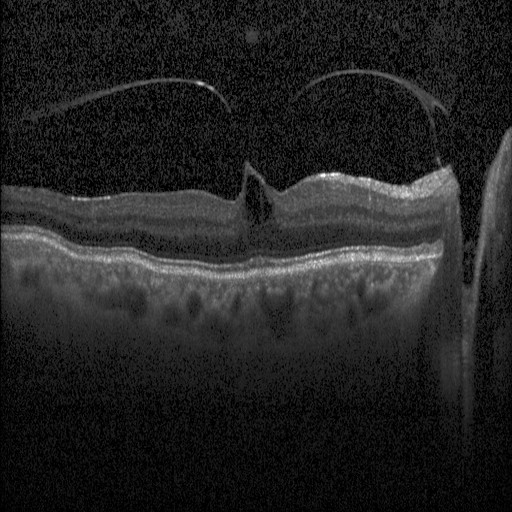
Spectral-domain OCT, through the macula, retinal OCT B-scan, acquired on a Heidelberg Spectralis
Impression: DME.